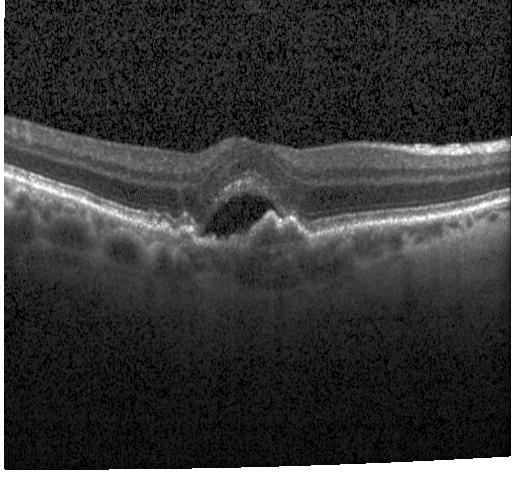

Centered on the fovea. Retinal OCT B-scan.
OCT finding: choroidal neovascularization (CNV).